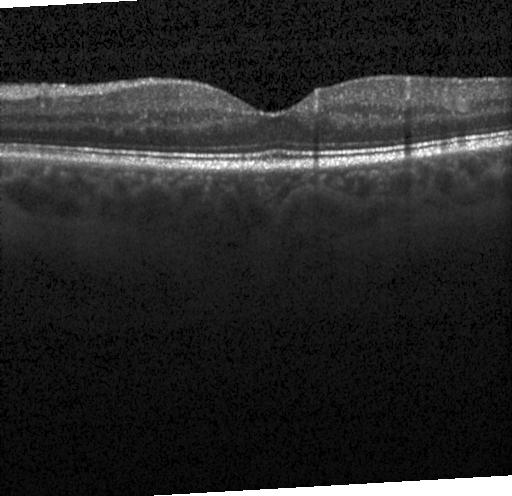
Macular OCT demonstrating no choroidal neovascularization, no diabetic macular edema, and no drusen.